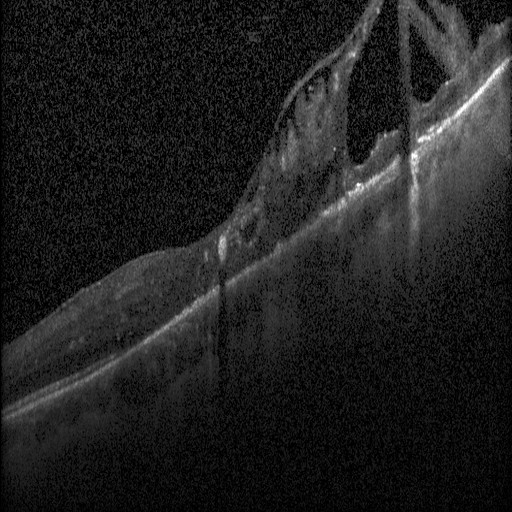 OCT B-scan; spectral-domain optical coherence tomography; through the macula; Heidelberg Spectralis OCT system — Assessment: DME.